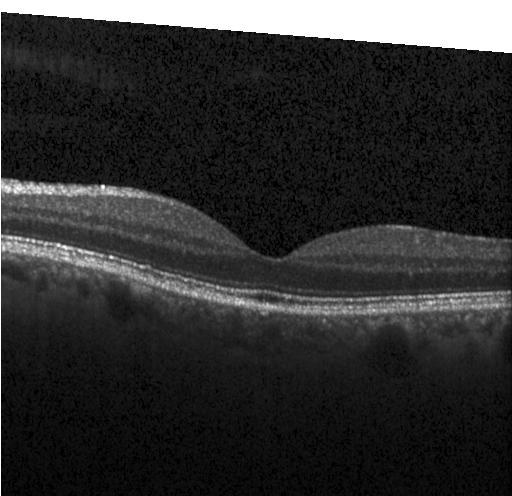

OCT B-scan. Dx: neither CNV, DME, nor drusen.